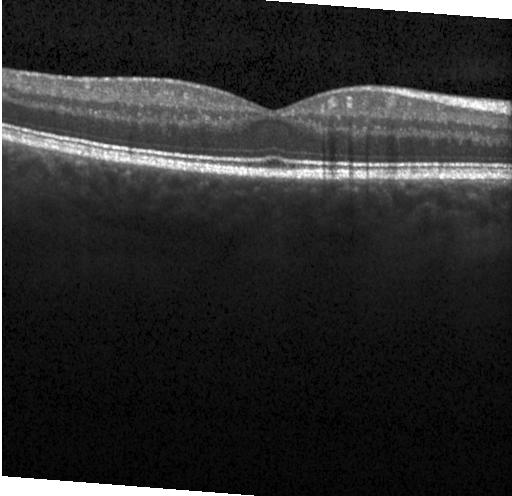 Acquired on a Heidelberg Spectralis; spectral-domain optical coherence tomography; optical coherence tomography scan.
Impression: no CNV, no DME, and no drusen.